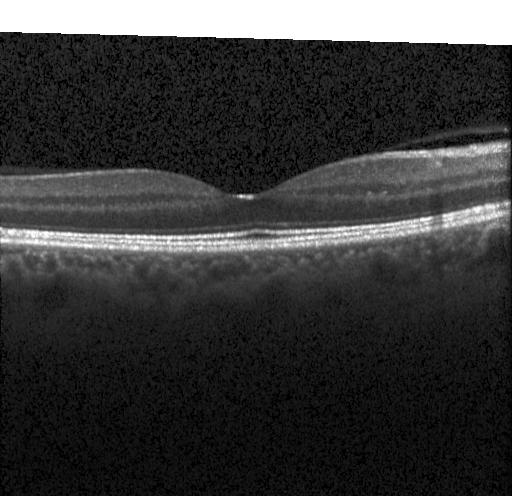

Heidelberg Spectralis, through the macula, OCT line scan
Impression: no choroidal neovascularization, no diabetic macular edema, and no drusen.